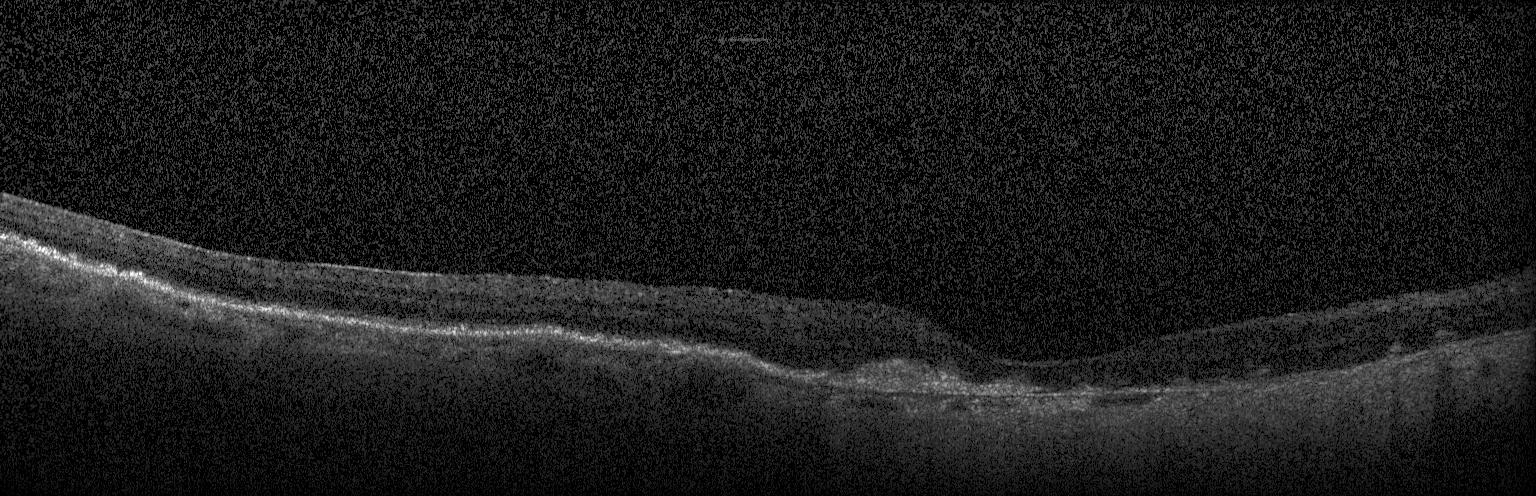

Retinal OCT cross-section.
This B-scan demonstrates choroidal neovascularization (CNV).